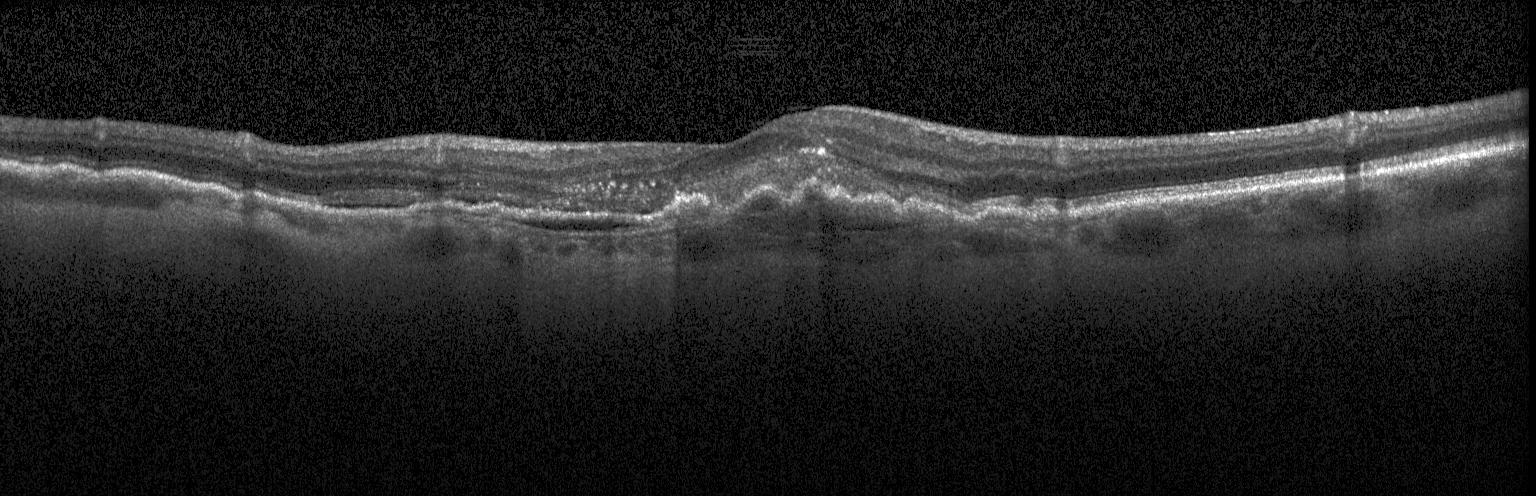 Retinal OCT B-scan
The scan shows choroidal neovascularization (CNV).